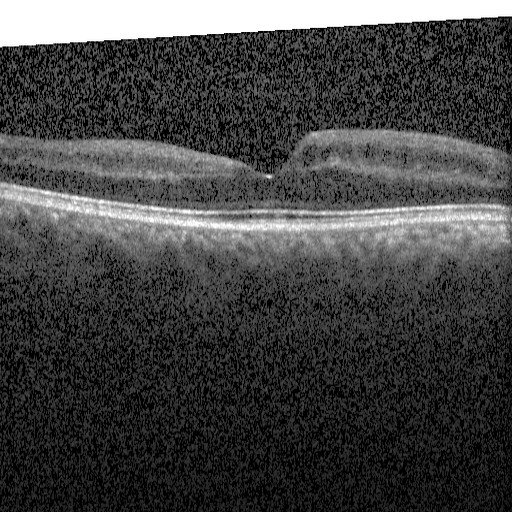

Finding: diabetic macular edema (DME).